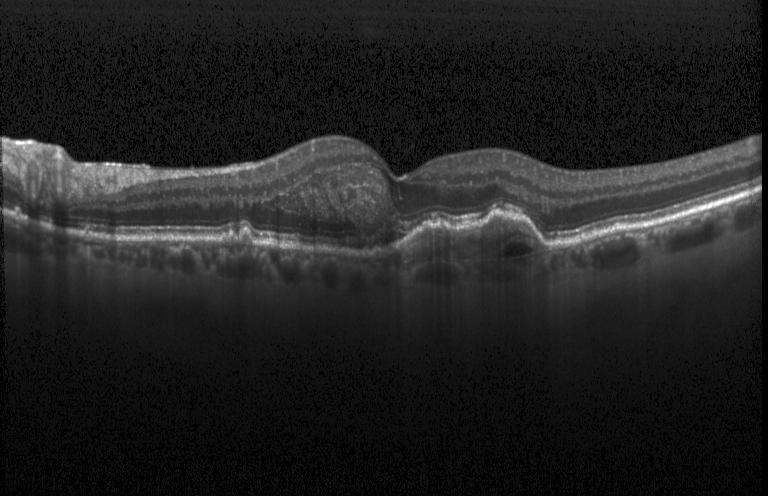

OCT line scan. Heidelberg Spectralis. SD-OCT. Horizontal scan through the fovea. Impression: a choroidal neovascular membrane.